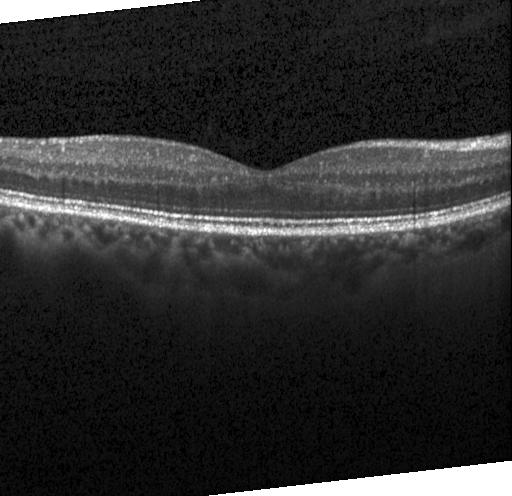 Impression: neither choroidal neovascularization, diabetic macular edema, nor drusen.